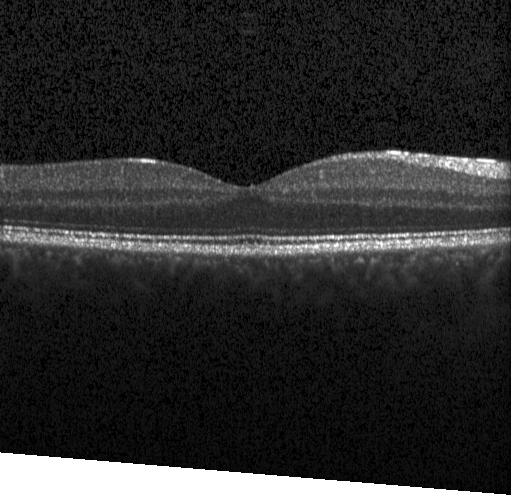
Finding: neither choroidal neovascularization, diabetic macular edema, nor drusen.